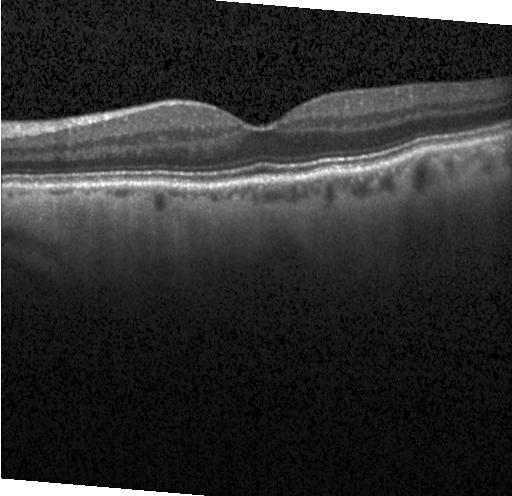
Optical coherence tomography B-scan.
Impression: no choroidal neovascularization, diabetic macular edema, or drusen.